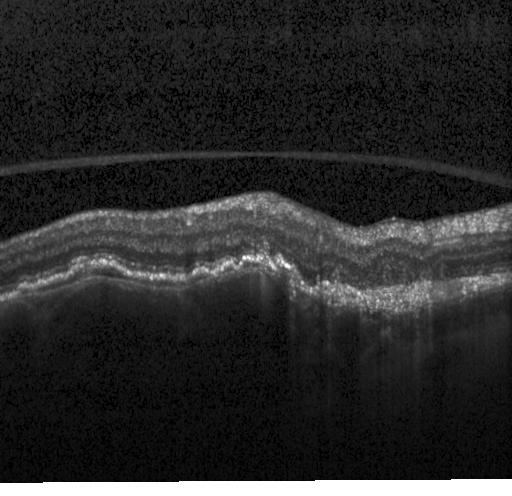

Finding: choroidal neovascularization.